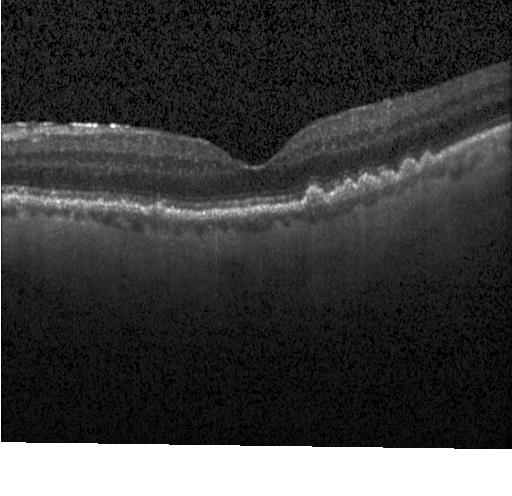
OCT scan showing drusen.